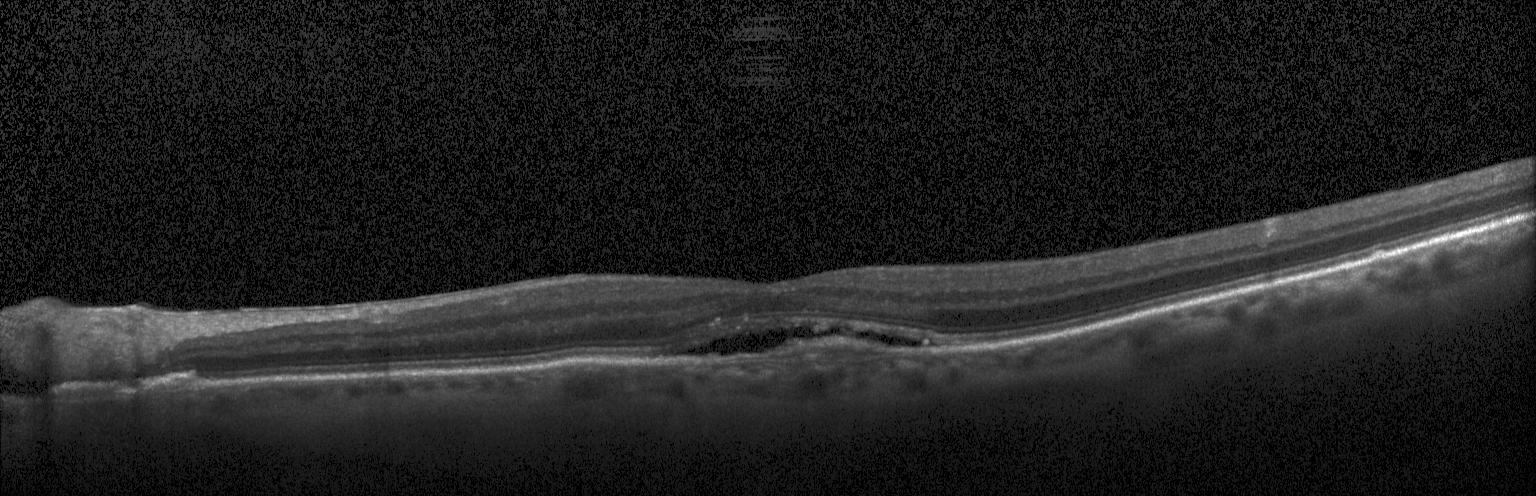

Fovea-centered. SD-OCT. Optical coherence tomography scan. Acquired on a Heidelberg Spectralis — Impression: choroidal neovascularization (CNV).